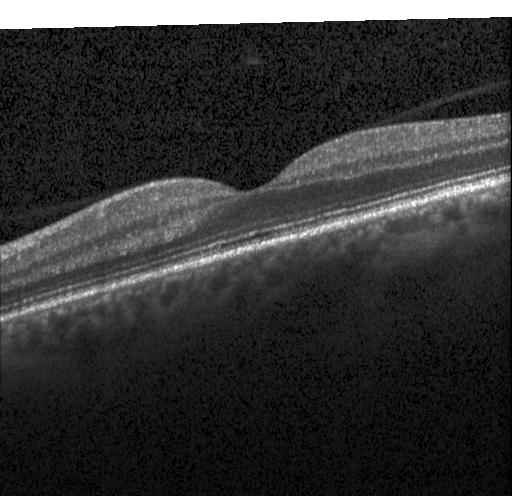
OCT line scan; Heidelberg Spectralis OCT system; spectral-domain OCT. Finding: neither choroidal neovascularization, diabetic macular edema, nor drusen.